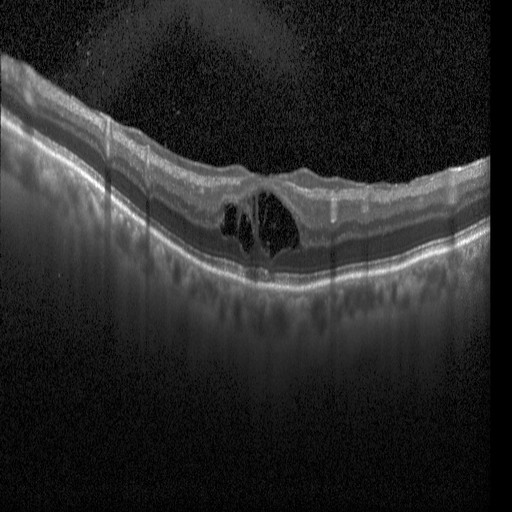
Finding: diabetic macular edema (DME).